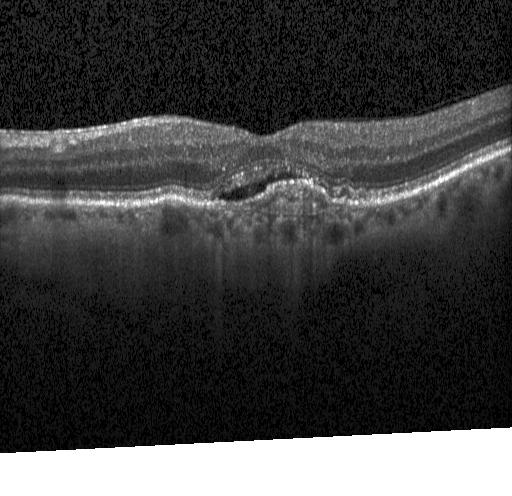
Retinal OCT B-scan · horizontal scan through the fovea · instrument: Heidelberg Spectralis.
The scan shows a choroidal neovascular membrane.